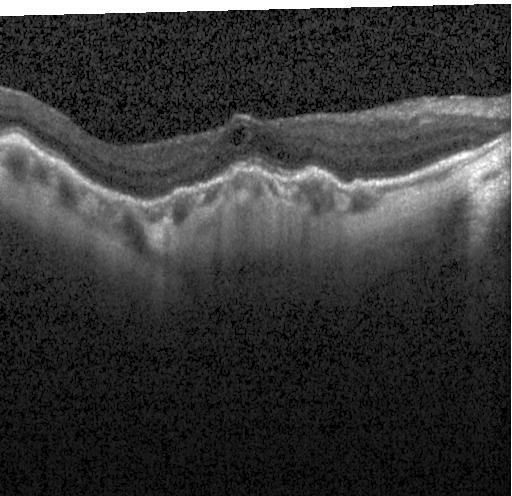 OCT finding: a choroidal neovascular membrane.